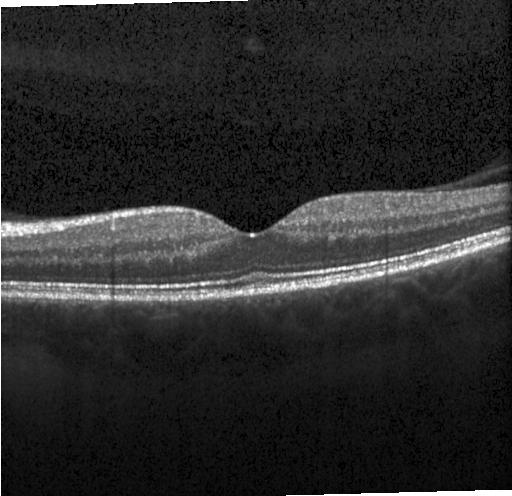
Macular scan · spectral-domain OCT · acquired on a Heidelberg Spectralis · OCT B-scan
Finding: neither choroidal neovascularization, diabetic macular edema, nor drusen.